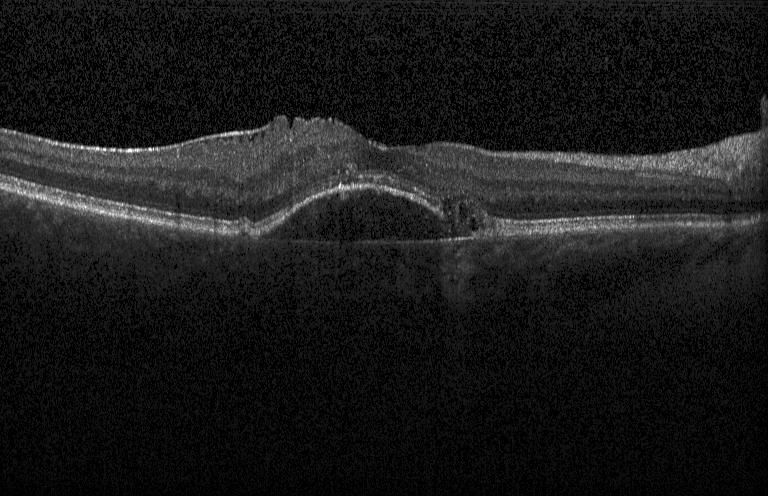 Retinal OCT B-scan, through the macula, Heidelberg Spectralis. This B-scan demonstrates choroidal neovascularization (CNV).